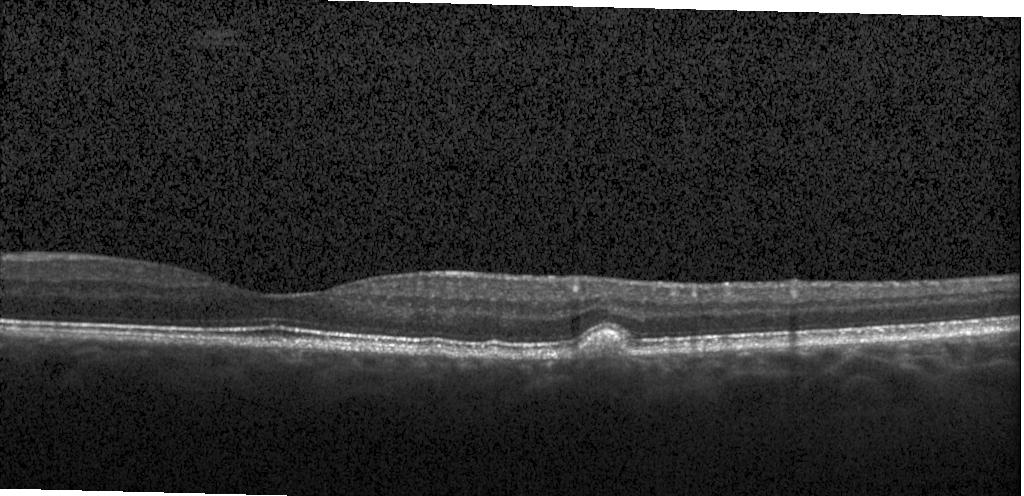 Optical coherence tomography scan · spectral-domain optical coherence tomography · Heidelberg Spectralis.
Diagnosis: sub-RPE drusenoid deposits.